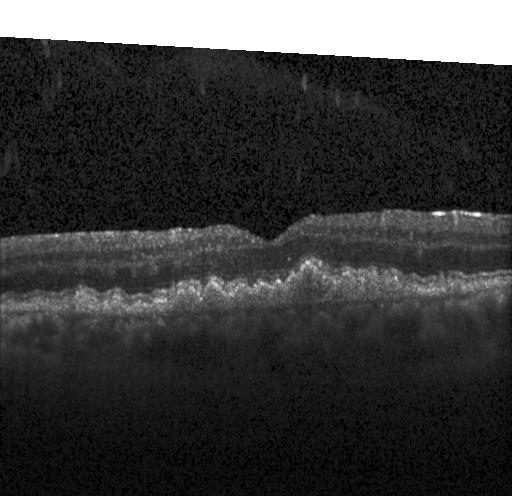
Heidelberg Spectralis OCT system. Horizontal scan through the fovea. Optical coherence tomography scan. Impression: a choroidal neovascular membrane.